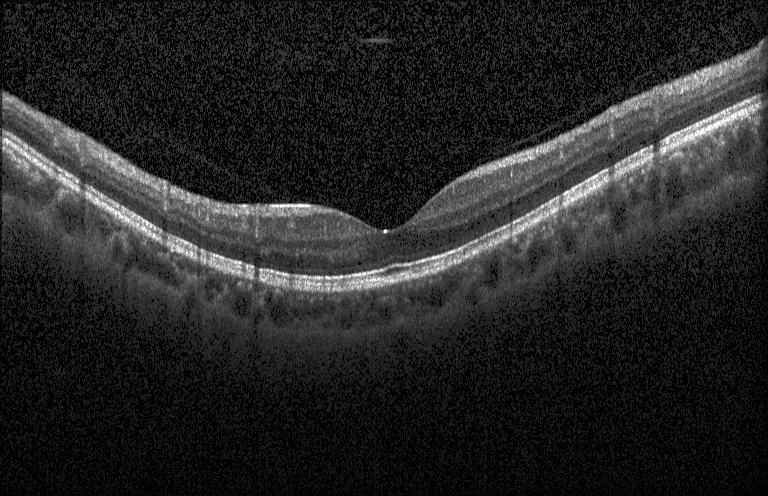

Optical coherence tomography B-scan.
This B-scan demonstrates neither choroidal neovascularization, diabetic macular edema, nor drusen.